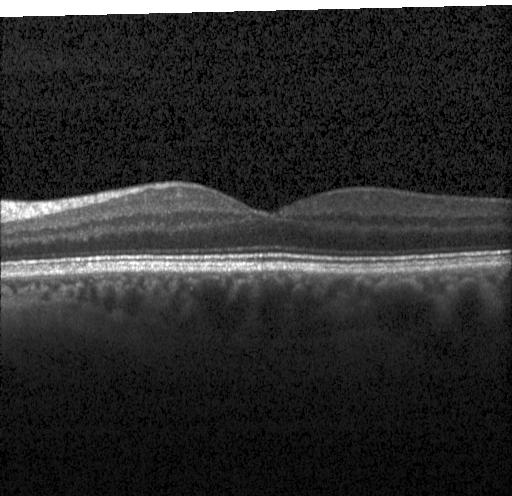 Finding: no CNV, DME, or drusen.